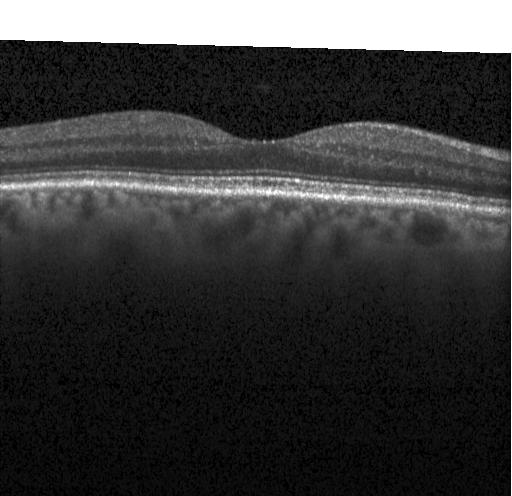
OCT line scan.
Diagnosis: no choroidal neovascularization, no diabetic macular edema, and no drusen.